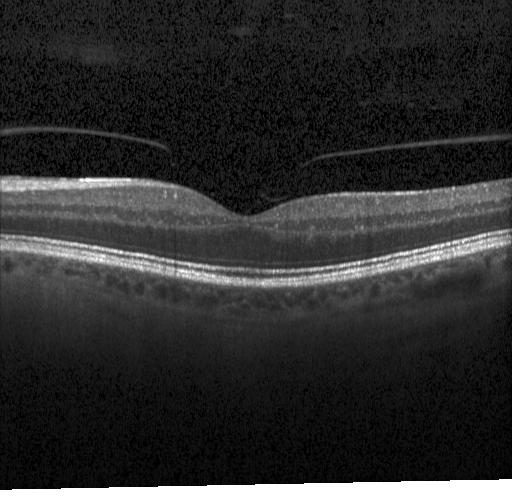

Diagnosis: neither choroidal neovascularization, diabetic macular edema, nor drusen.